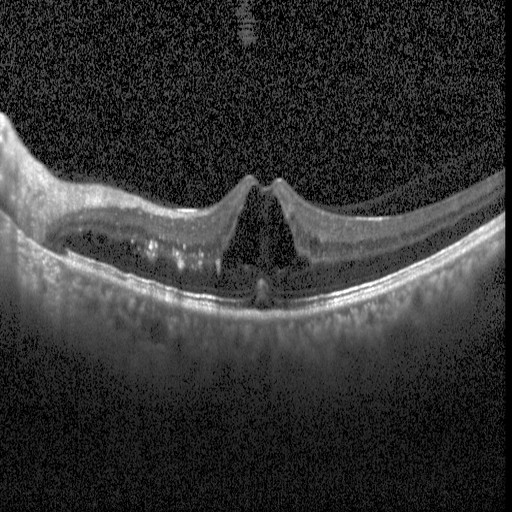
OCT line scan.
Finding: diabetic macular edema (DME).